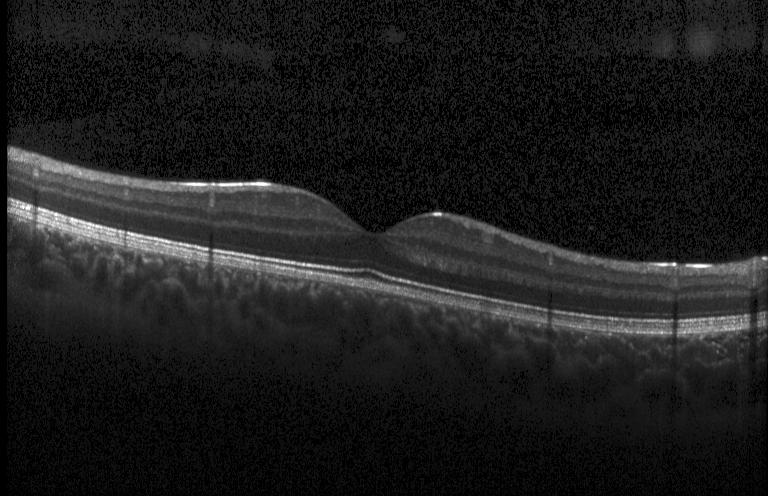

OCT B-scan showing no choroidal neovascularization, diabetic macular edema, or drusen.